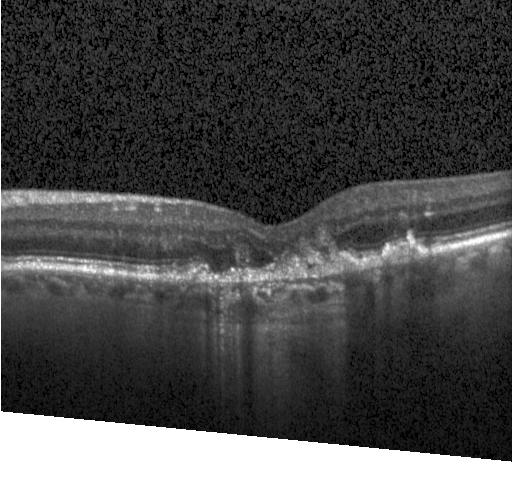
Diagnosis: a choroidal neovascular membrane.